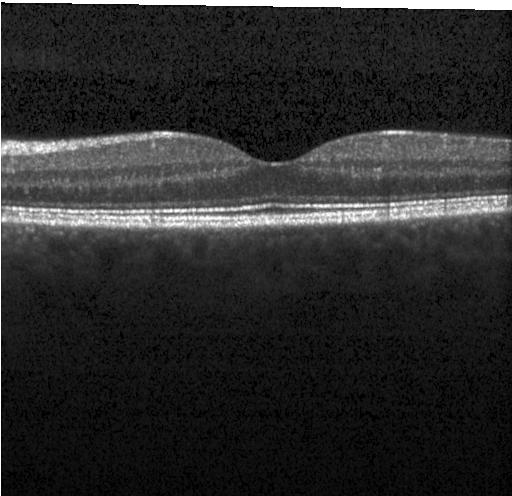

This B-scan demonstrates no evidence of choroidal neovascularization, diabetic macular edema, or drusen.